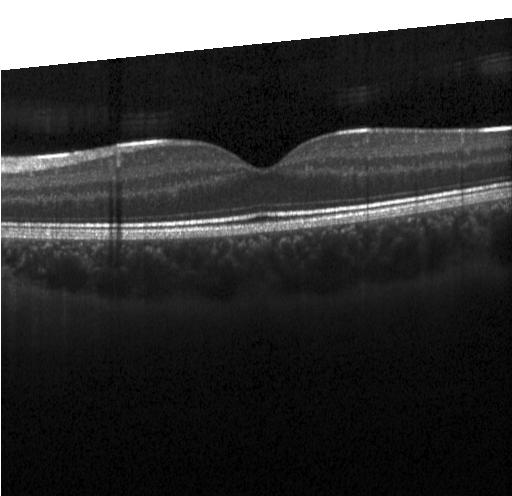
Fovea-centered; optical coherence tomography scan; Heidelberg Spectralis OCT system; spectral-domain optical coherence tomography
Finding: no evidence of choroidal neovascularization, diabetic macular edema, or drusen.